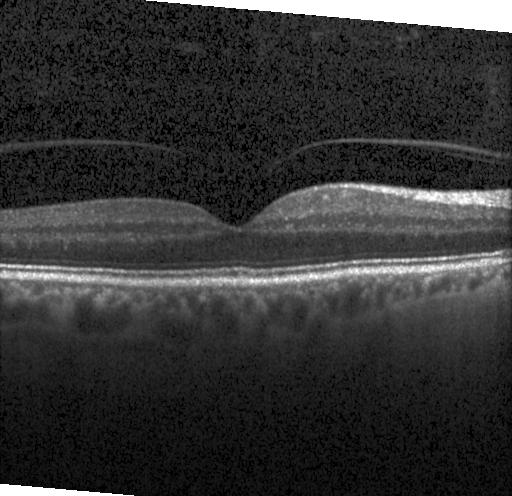 Spectral-domain optical coherence tomography · retinal OCT B-scan · Heidelberg Spectralis OCT system. Diagnosis: neither CNV, DME, nor drusen.